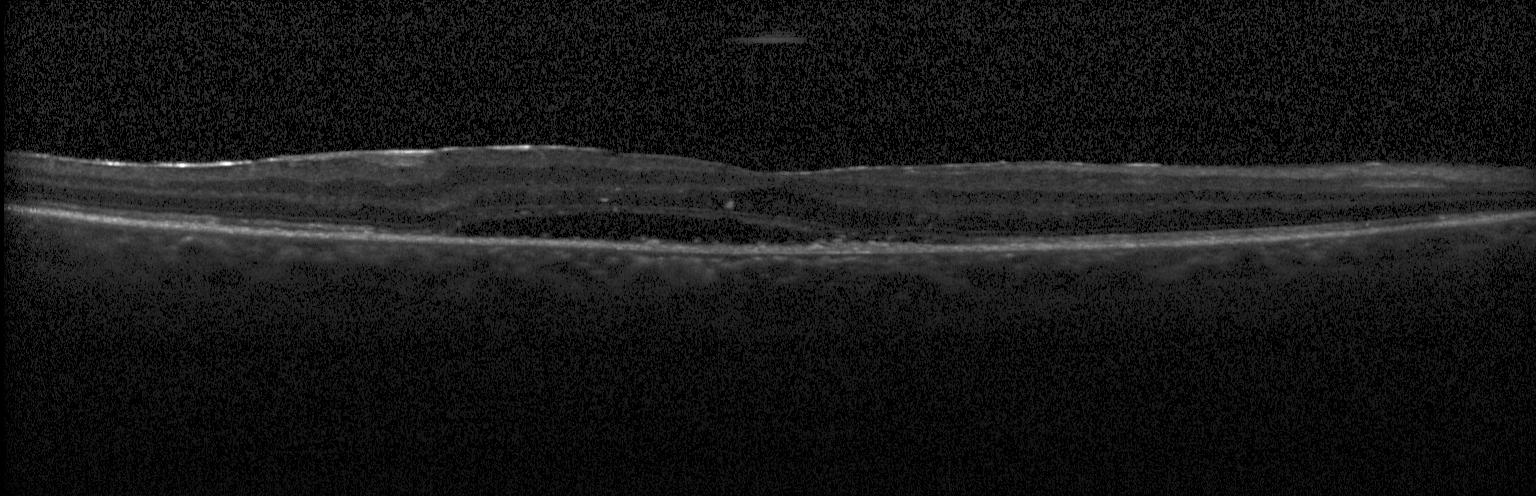

Finding: a choroidal neovascular membrane.